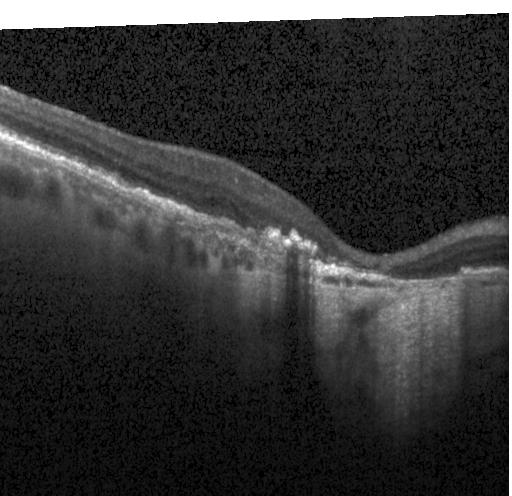
OCT finding: CNV.